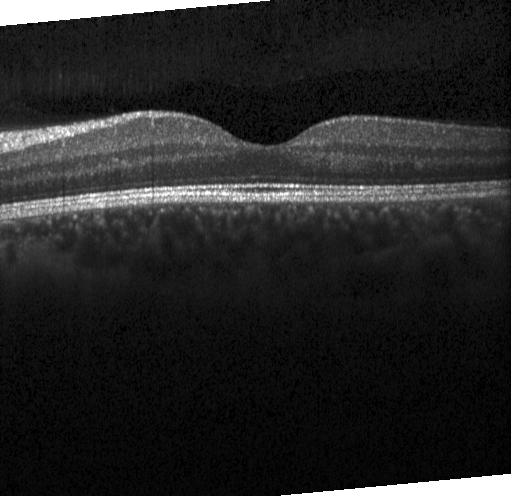

This B-scan demonstrates no CNV, no DME, and no drusen.